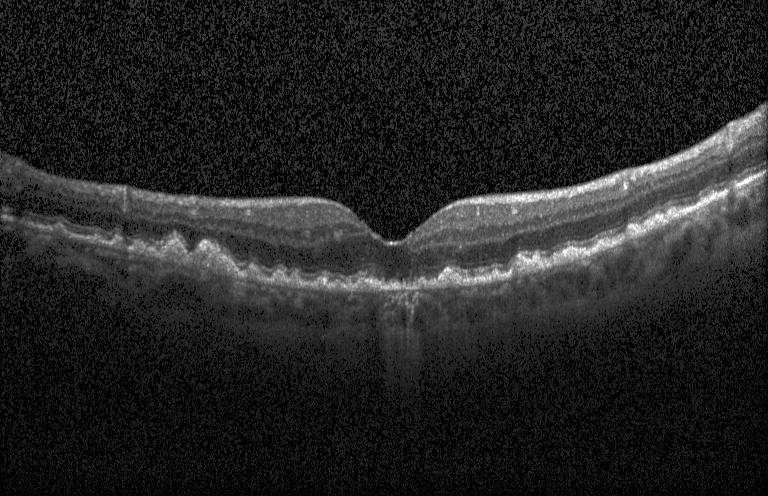
Finding: multiple drusen.